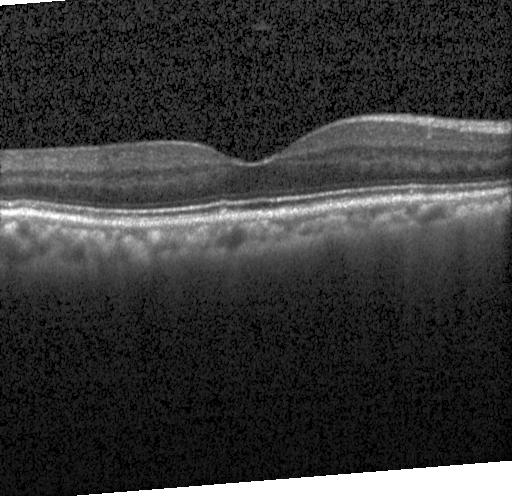 OCT B-scan — This B-scan demonstrates neither choroidal neovascularization, diabetic macular edema, nor drusen.